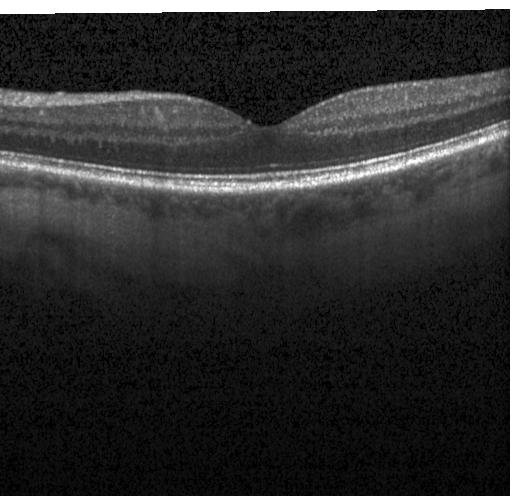

Optical coherence tomography scan
Assessment: neither choroidal neovascularization, diabetic macular edema, nor drusen.